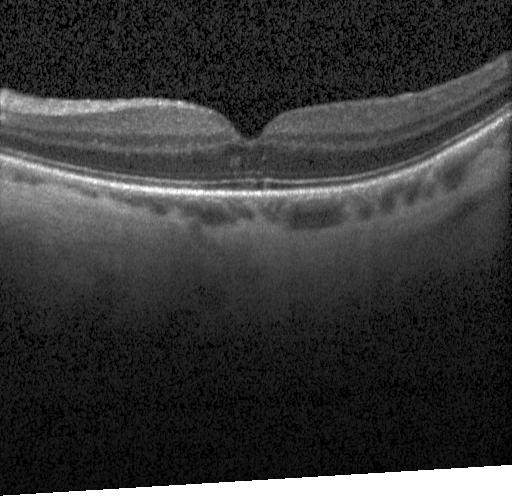 OCT line scan, Heidelberg Spectralis. OCT finding: diabetic macular edema.